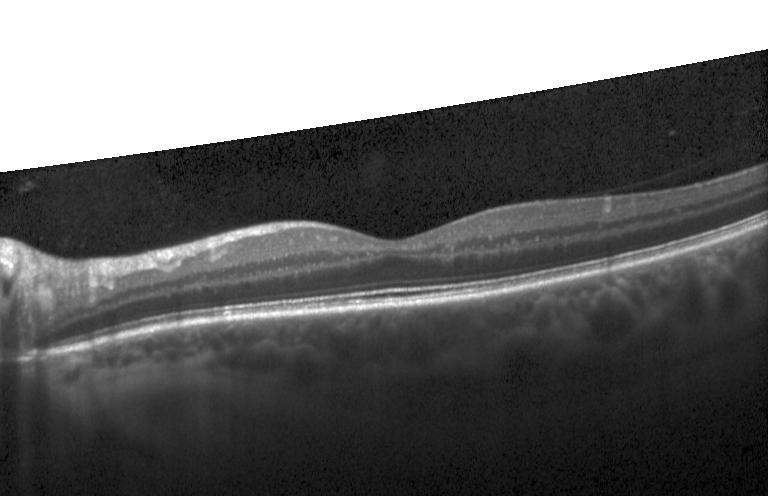

Macular OCT demonstrating no choroidal neovascularization, diabetic macular edema, or drusen.